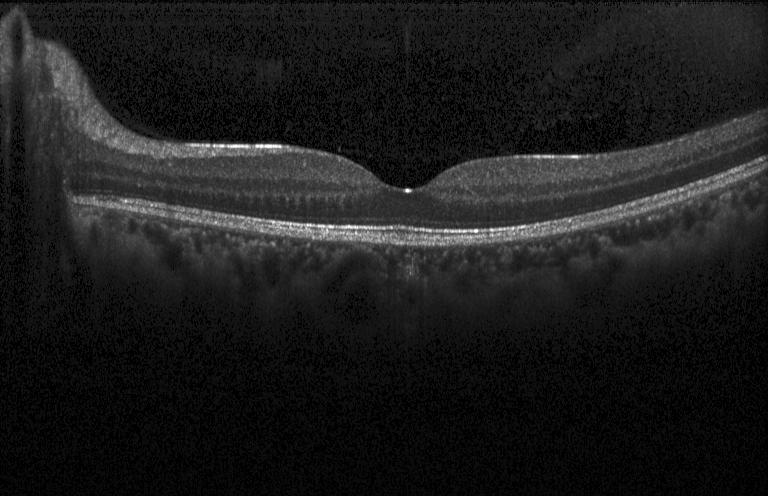 Optical coherence tomography scan.
OCT finding: no CNV, DME, or drusen.